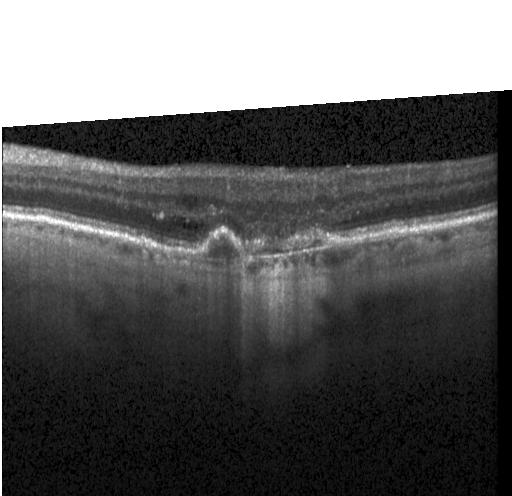
Horizontal scan through the fovea. OCT B-scan
Choroidal neovascularization.